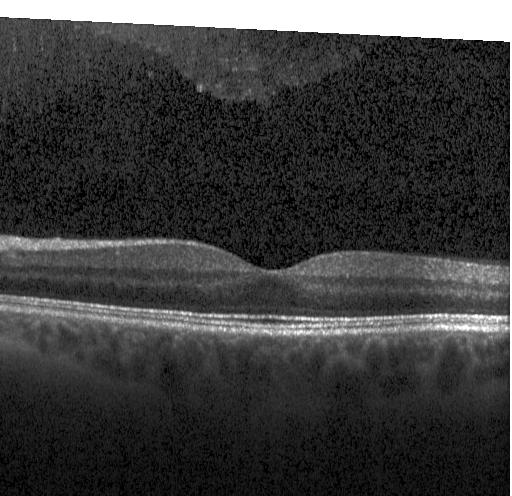
OCT scan showing no evidence of CNV, DME, or drusen.